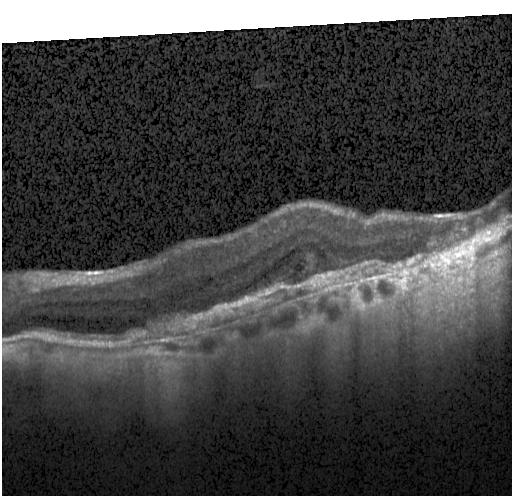 OCT scan showing choroidal neovascularization.